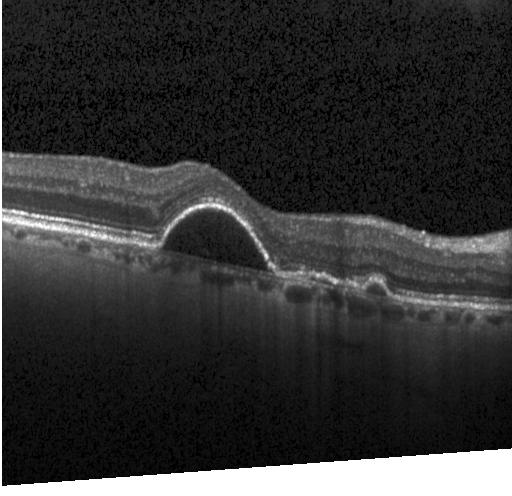 SD-OCT, retinal OCT cross-section
Assessment: a choroidal neovascular membrane.